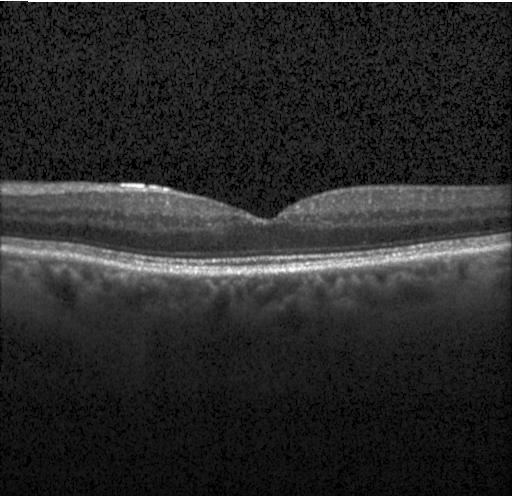
OCT B-scan — Dx: no choroidal neovascularization, diabetic macular edema, or drusen.